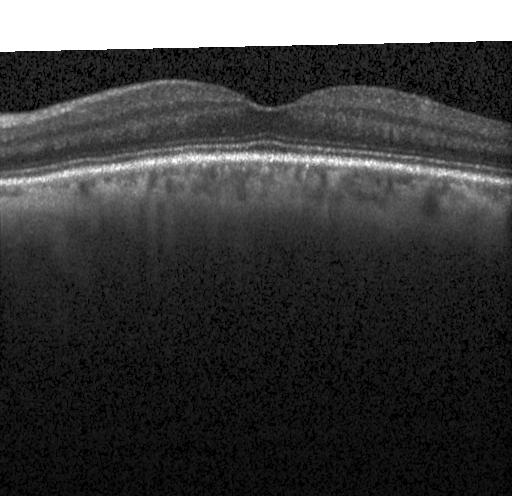
Optical coherence tomography B-scan. This B-scan demonstrates neither choroidal neovascularization, diabetic macular edema, nor drusen.